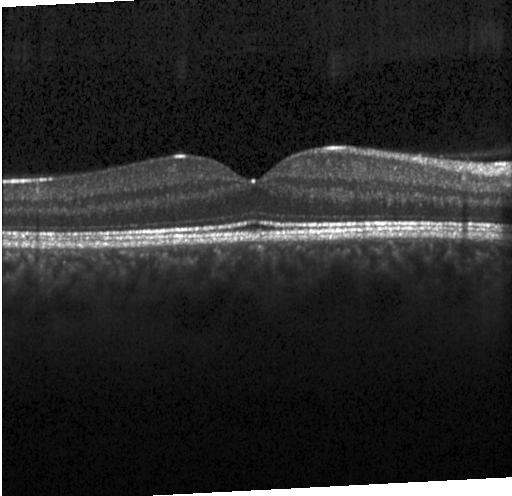 OCT scan showing no evidence of choroidal neovascularization, diabetic macular edema, or drusen.